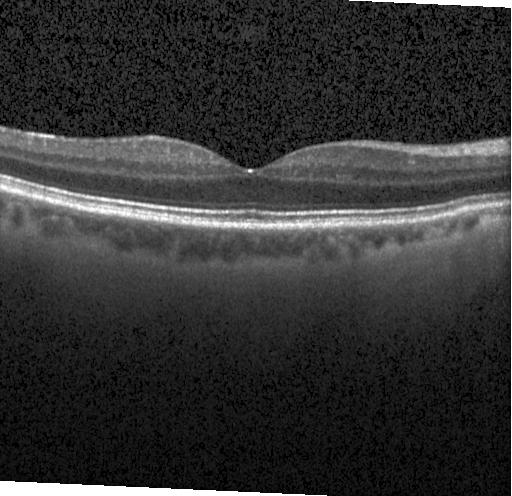 Optical coherence tomography scan.
OCT finding: no evidence of choroidal neovascularization, diabetic macular edema, or drusen.